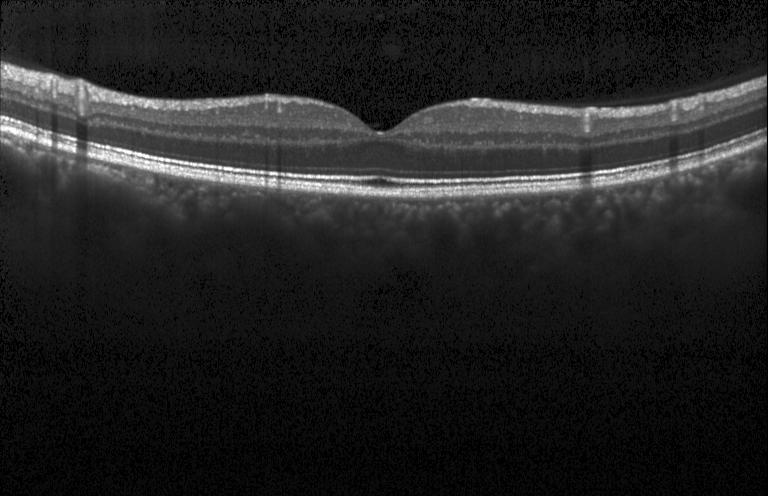 SD-OCT; fovea-centered; optical coherence tomography B-scan.
Macular OCT: no CNV, no DME, and no drusen.